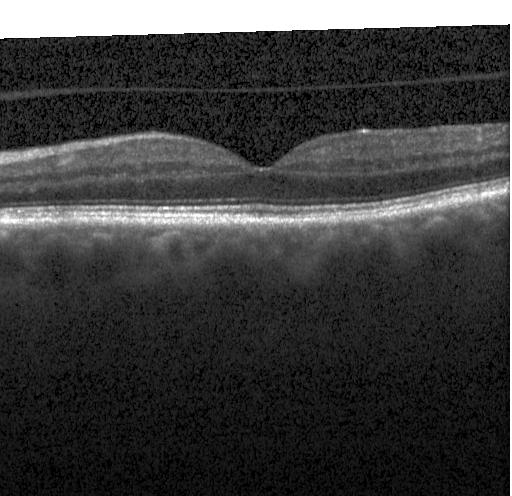
Diagnosis: no choroidal neovascularization, diabetic macular edema, or drusen.